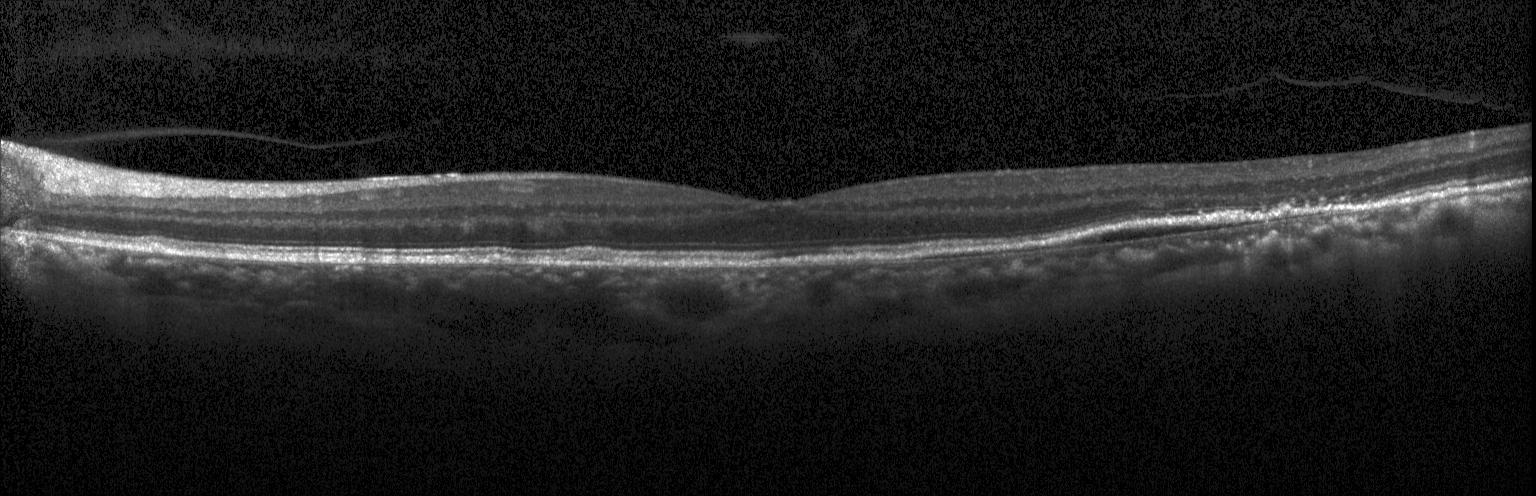

Diagnosis: a choroidal neovascular membrane.